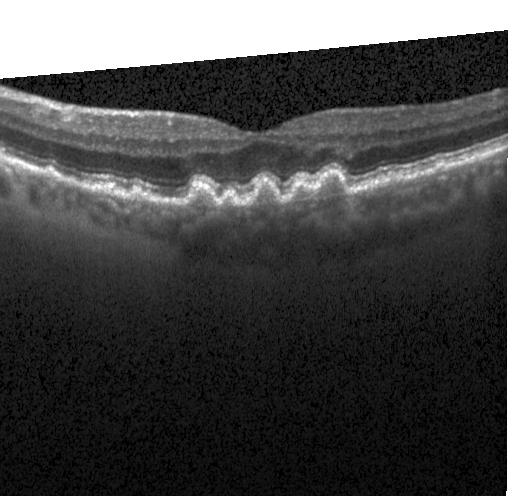
OCT B-scan showing multiple drusen.